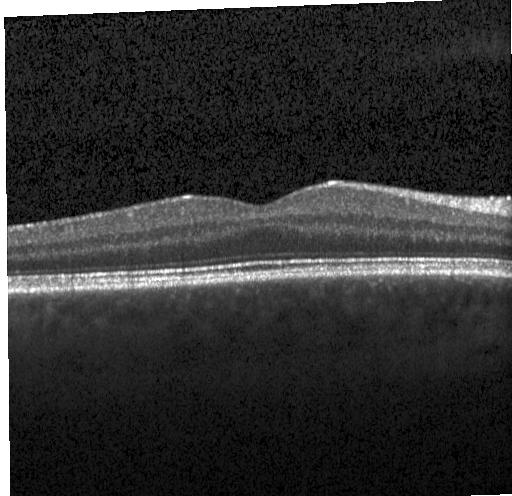

Impression: no choroidal neovascularization, diabetic macular edema, or drusen.